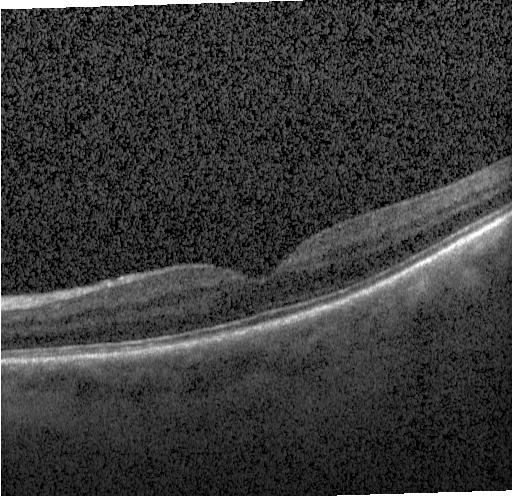 Finding: no choroidal neovascularization, no diabetic macular edema, and no drusen.